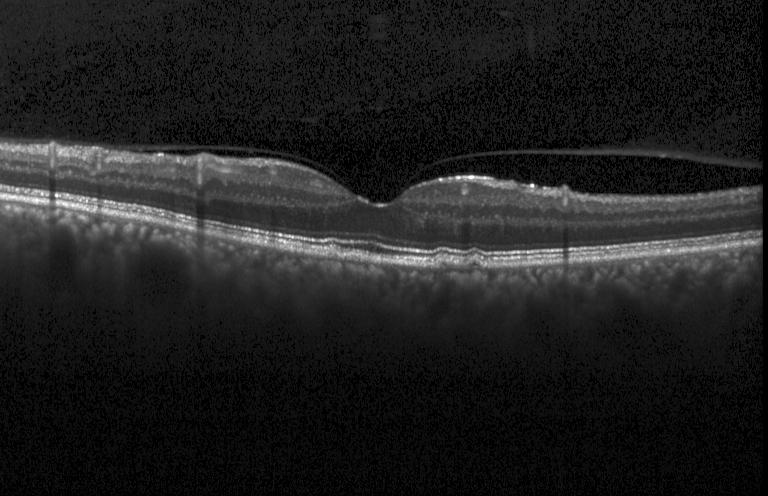
Finding: multiple drusen.